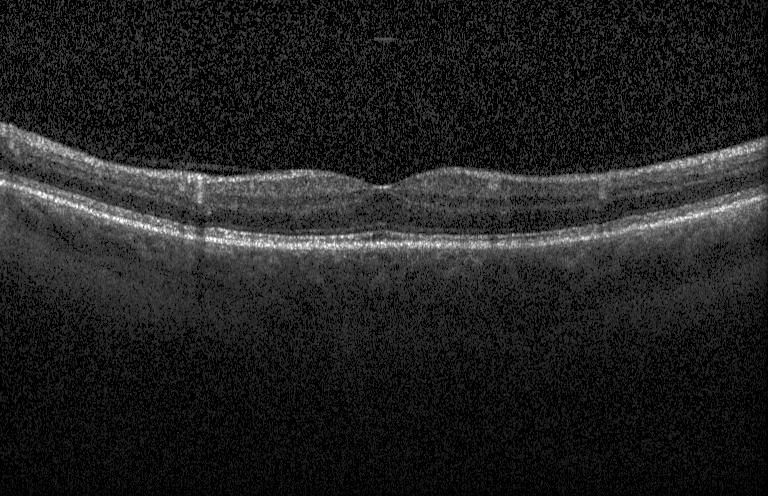

Retinal OCT cross-section, Heidelberg Spectralis OCT system.
Neither CNV, DME, nor drusen.